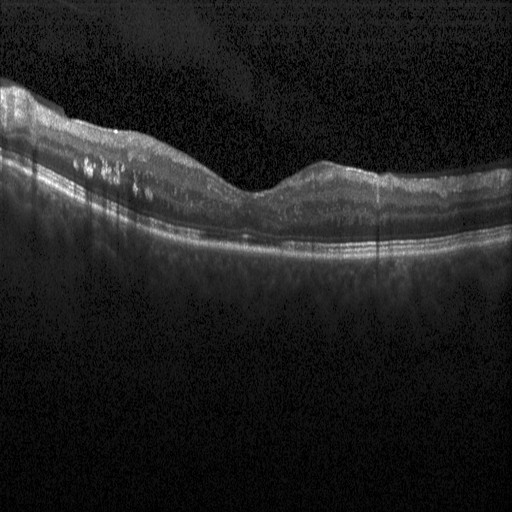
Macular scan · retinal OCT cross-section · SD-OCT · instrument: Heidelberg Spectralis. Assessment: diabetic macular edema (DME).